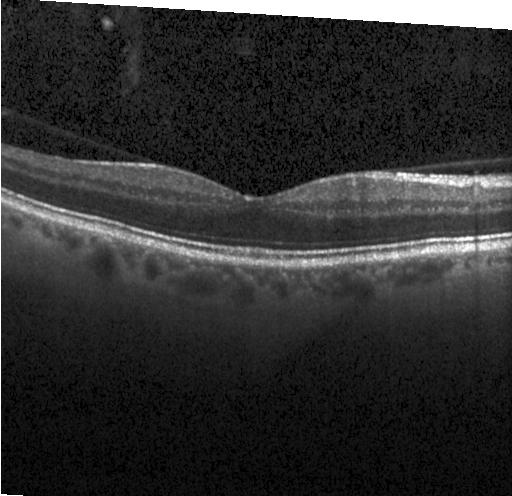

OCT B-scan. Heidelberg Spectralis OCT system. Spectral-domain optical coherence tomography. Through the macula.
This B-scan demonstrates no CNV, no DME, and no drusen.